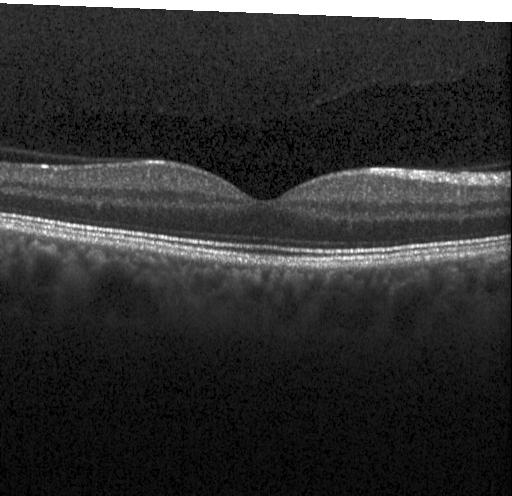 Retinal OCT cross-section; spectral-domain optical coherence tomography; through the macula. Dx: no CNV, no DME, and no drusen.